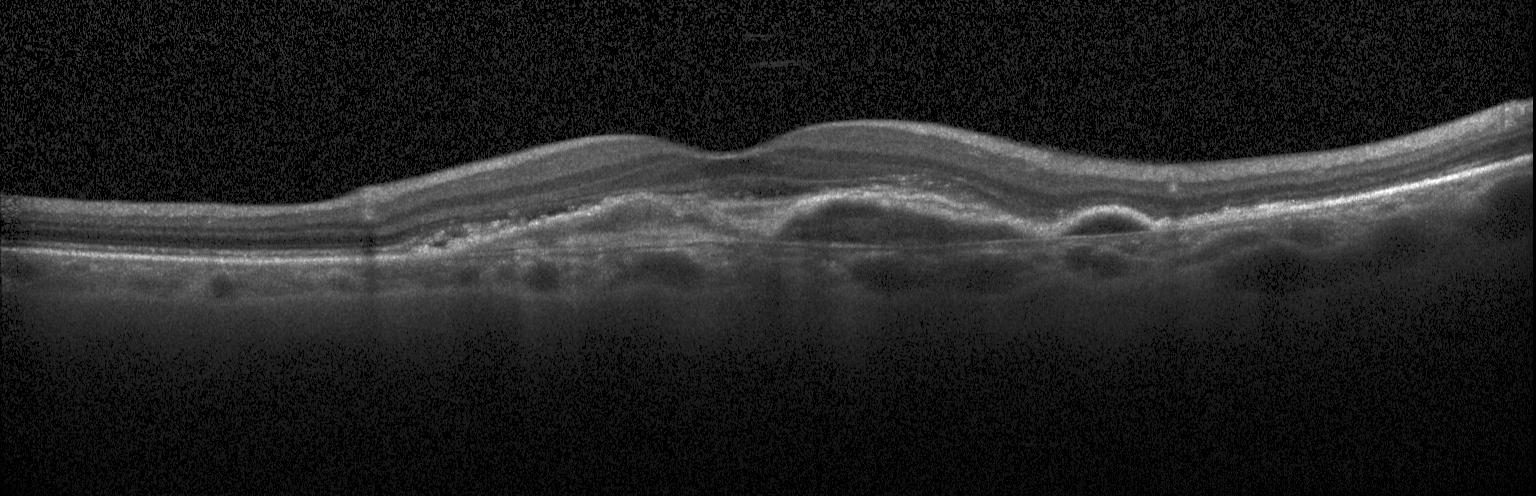 Optical coherence tomography B-scan
Finding: a choroidal neovascular membrane.